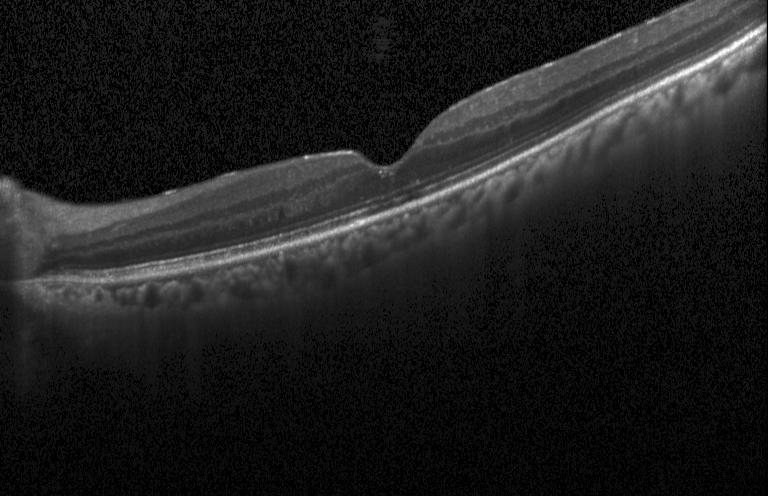
Centered on the fovea · OCT line scan
Impression: neither choroidal neovascularization, diabetic macular edema, nor drusen.